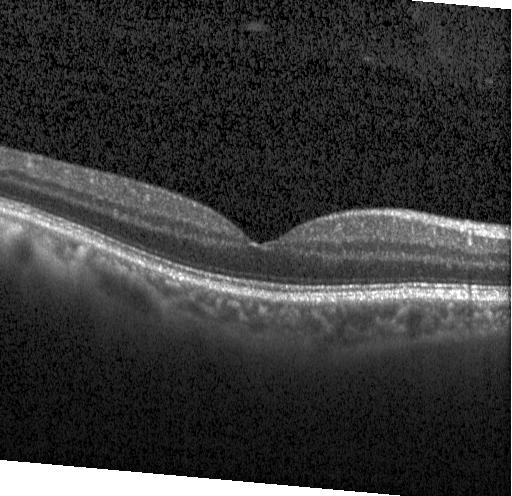

Heidelberg Spectralis OCT system. SD-OCT. Retinal OCT cross-section. Through the macula.
Neither CNV, DME, nor drusen.